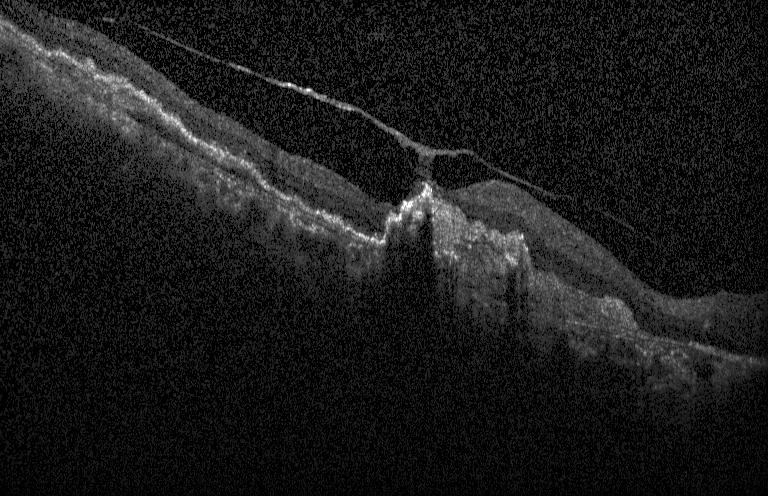 Macular OCT: a choroidal neovascular membrane.